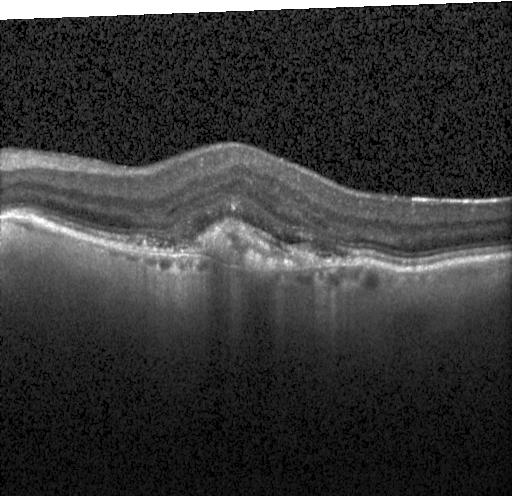
OCT scan showing choroidal neovascularization.